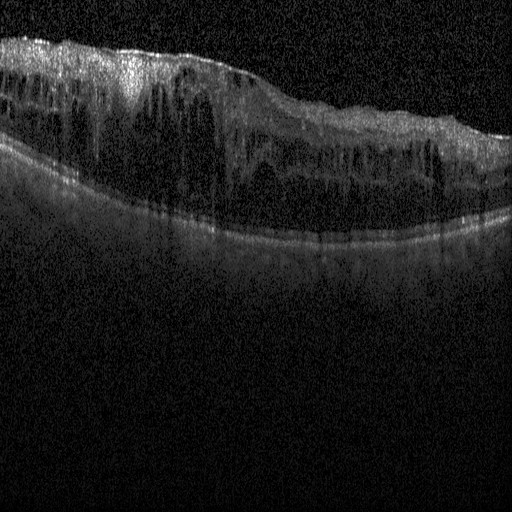 Optical coherence tomography scan.
Diagnosis: DME.